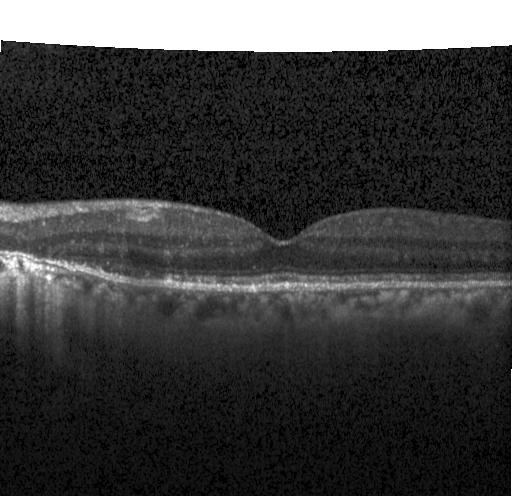
Optical coherence tomography B-scan · spectral-domain optical coherence tomography.
Diagnosis: no evidence of choroidal neovascularization, diabetic macular edema, or drusen.